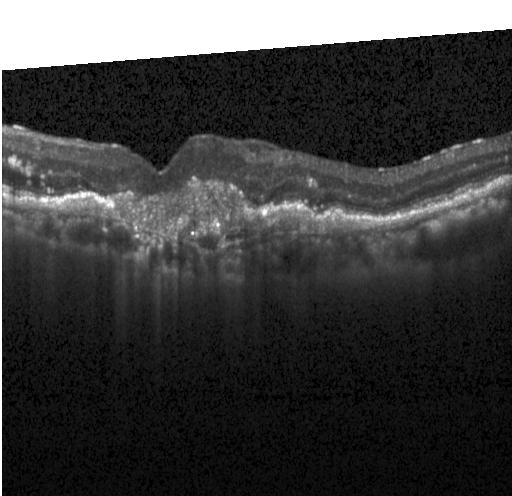

OCT line scan. The scan shows a choroidal neovascular membrane.